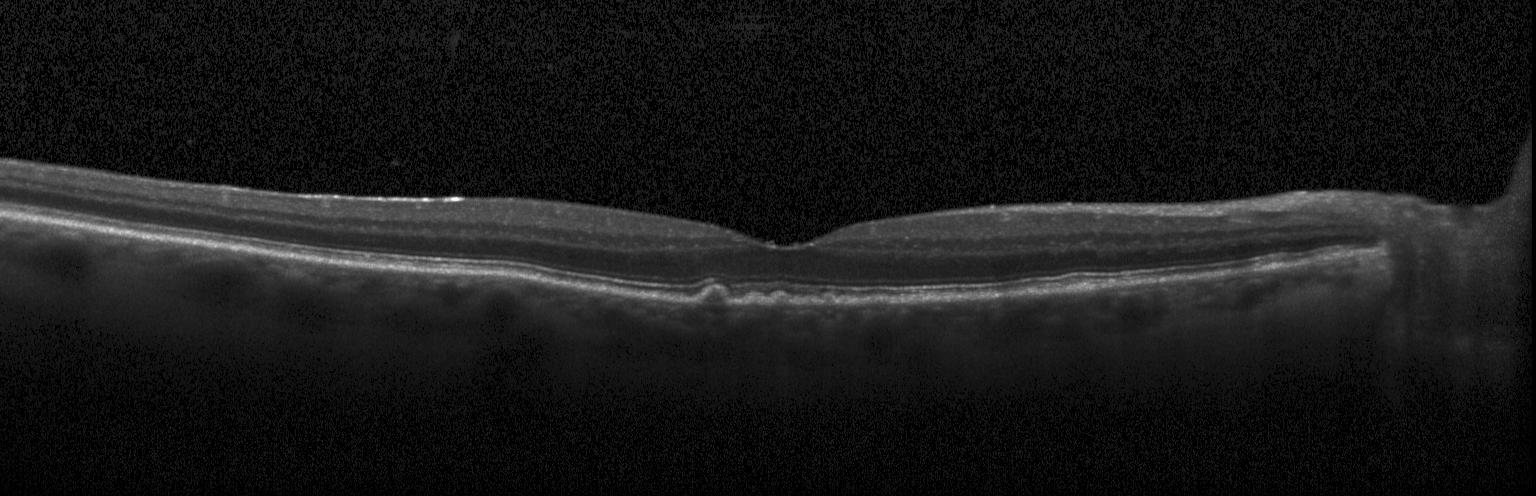
Finding: drusen.